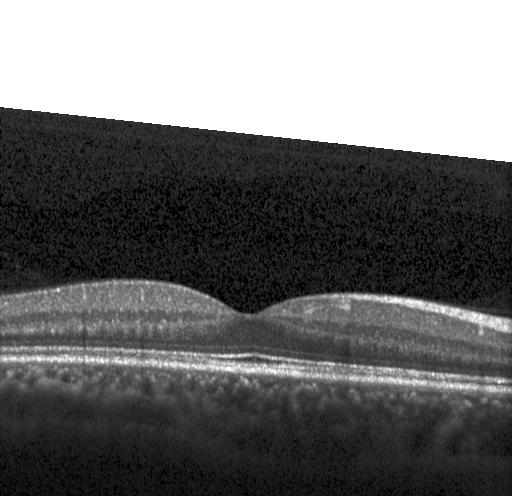 OCT B-scan showing neither choroidal neovascularization, diabetic macular edema, nor drusen.